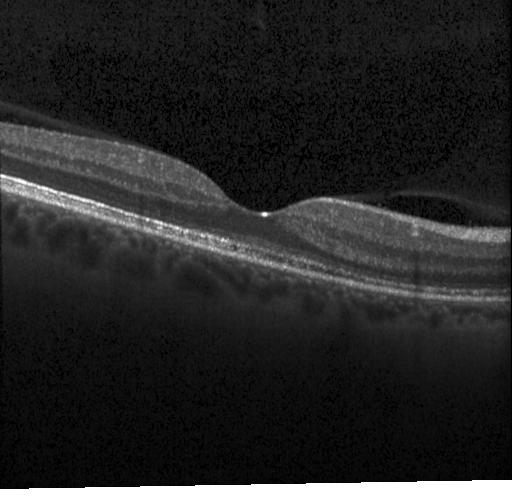
Optical coherence tomography B-scan.
Finding: neither CNV, DME, nor drusen.